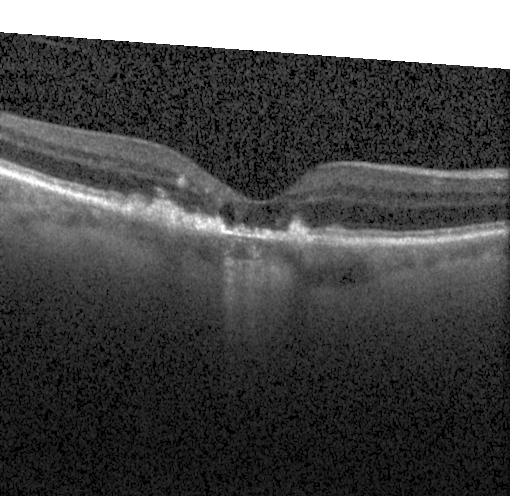 The scan shows a choroidal neovascular membrane.